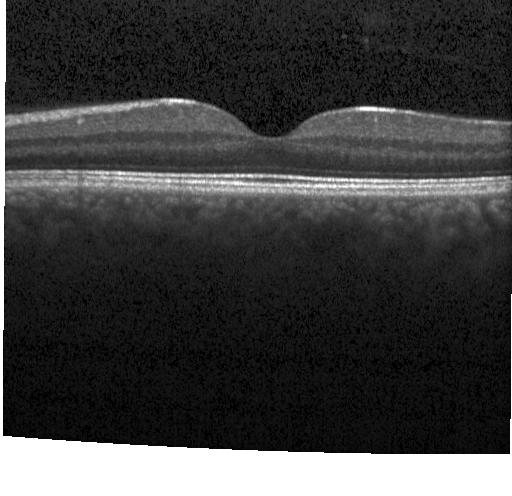
Heidelberg Spectralis. Retinal OCT B-scan — Diagnosis: no CNV, DME, or drusen.